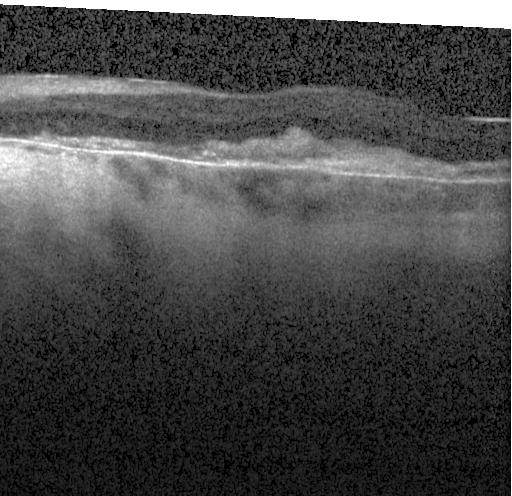

Fovea-centered, retinal OCT B-scan, spectral-domain optical coherence tomography
A choroidal neovascular membrane.